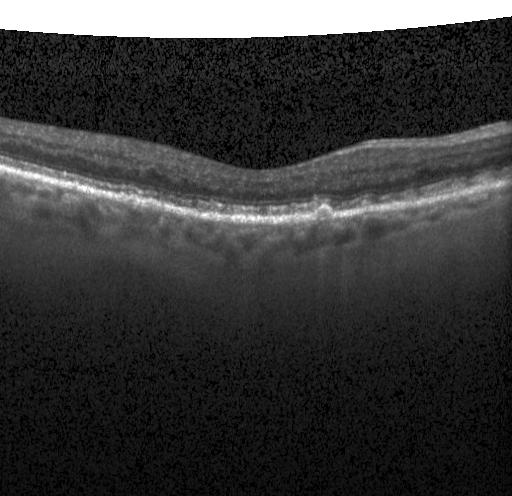
Diagnosis: drusen.